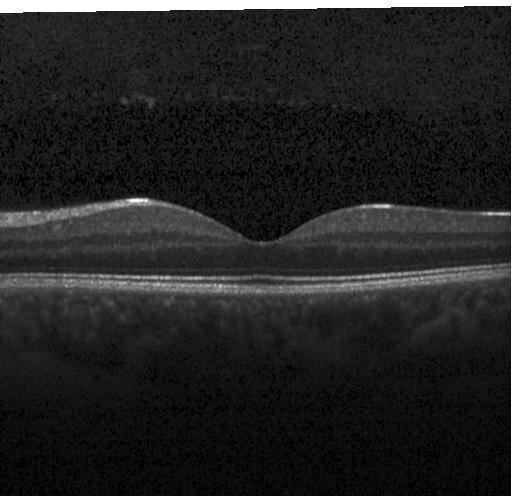 Finding: no evidence of choroidal neovascularization, diabetic macular edema, or drusen.